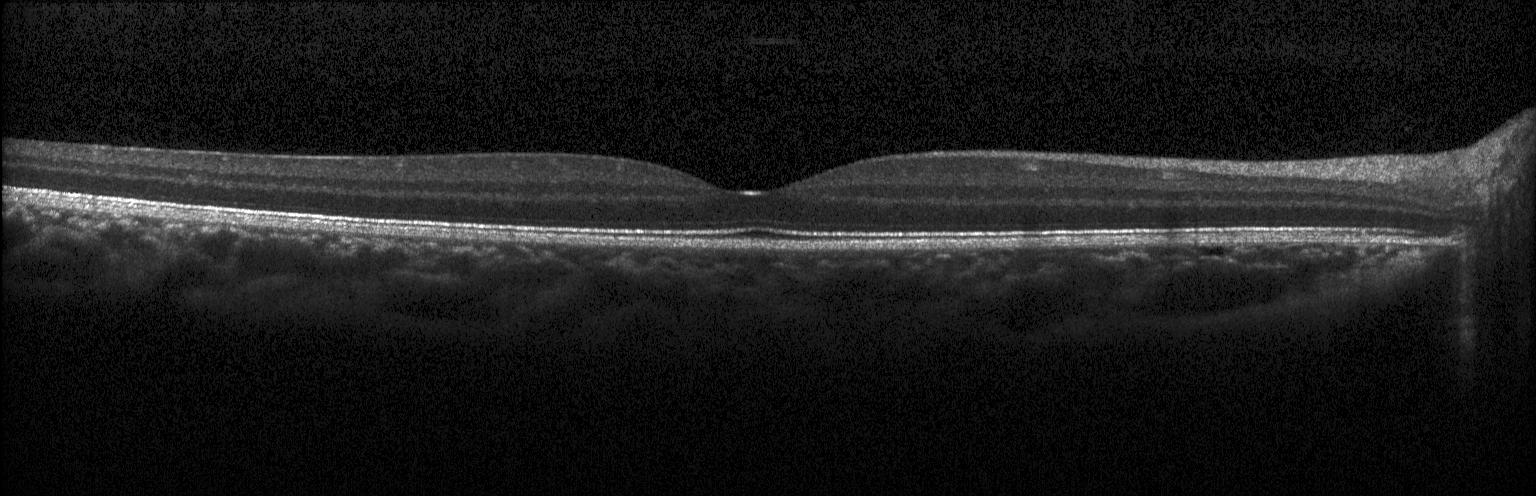

Heidelberg Spectralis, fovea-centered, OCT line scan — Diagnosis: no choroidal neovascularization, no diabetic macular edema, and no drusen.